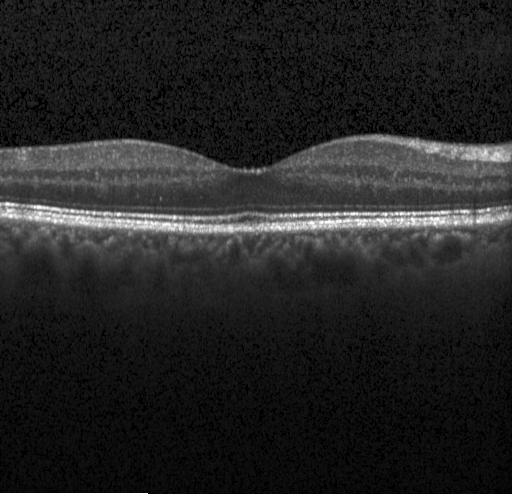

OCT B-scan.
This B-scan demonstrates no choroidal neovascularization, diabetic macular edema, or drusen.